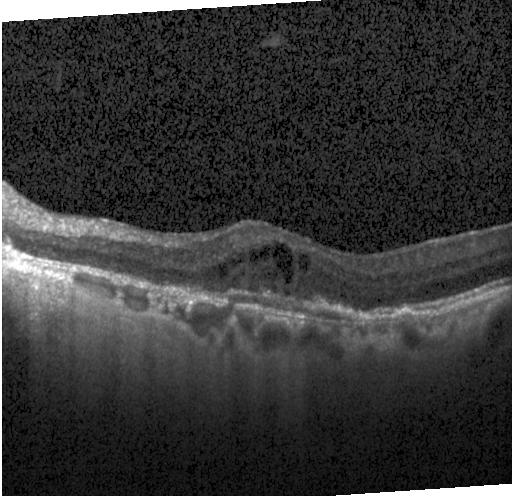
Optical coherence tomography scan; centered on the fovea. Dx: a choroidal neovascular membrane.